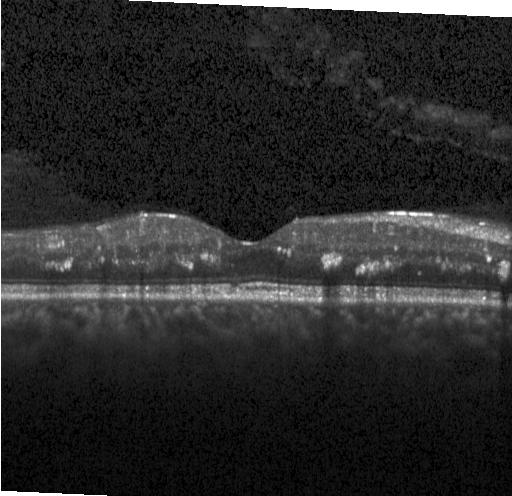 Spectral-domain OCT B-scan: diabetic macular edema (DME).